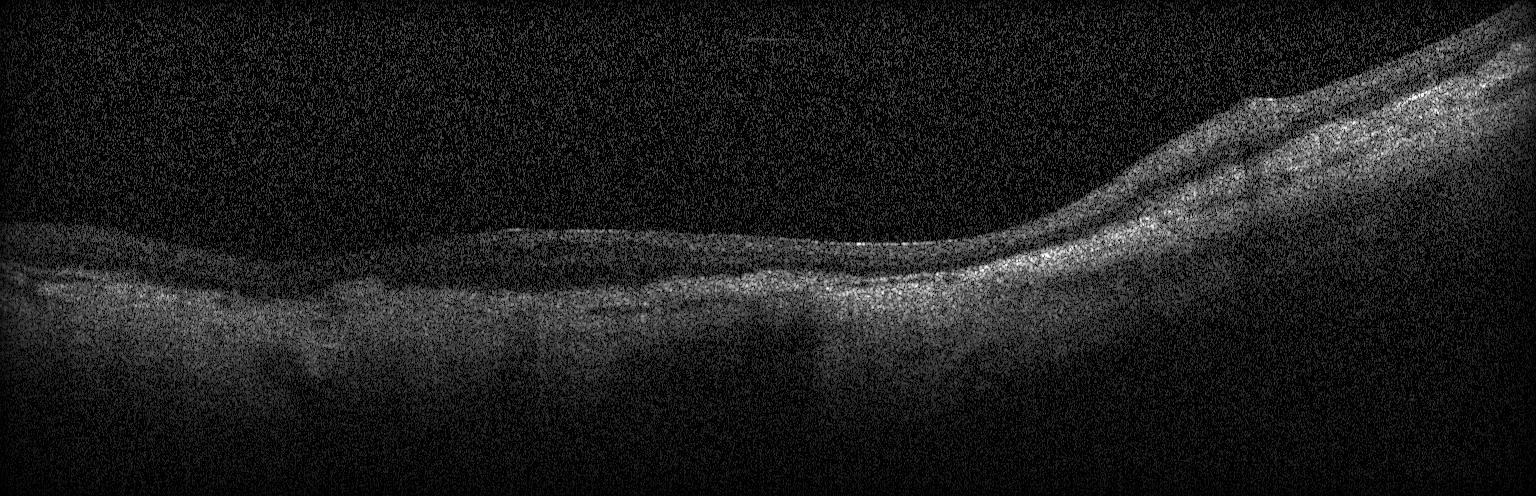 Spectral-domain optical coherence tomography, OCT line scan, horizontal scan through the fovea.
Impression: a choroidal neovascular membrane.